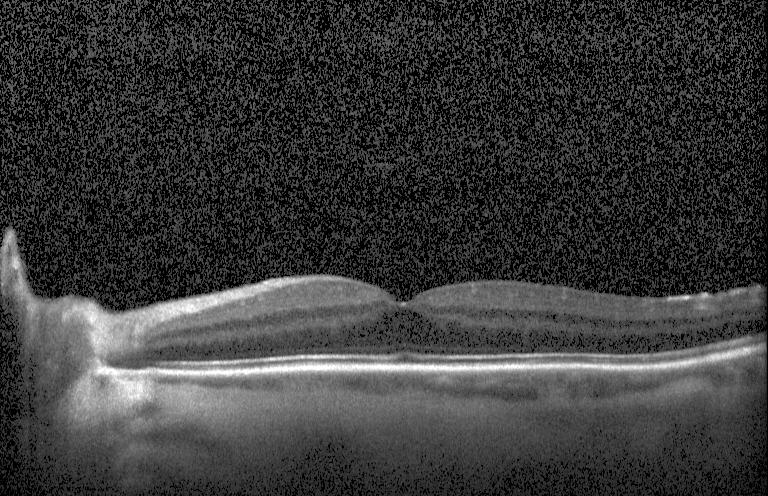 OCT line scan
The scan shows no CNV, DME, or drusen.